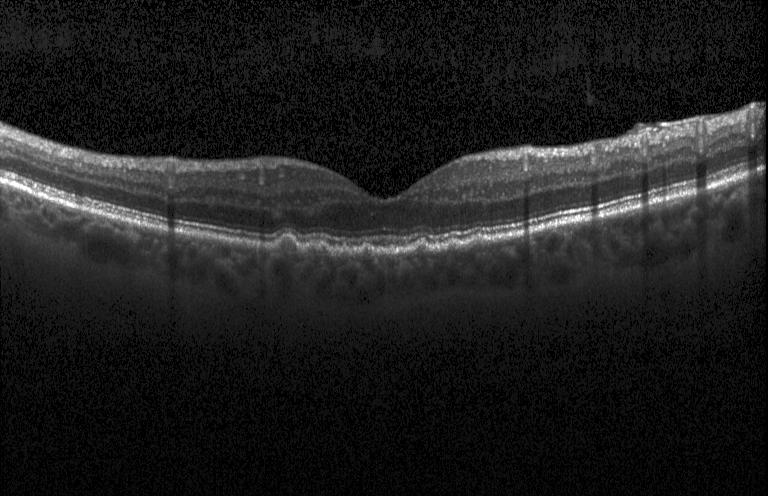

Optical coherence tomography scan; acquired on a Heidelberg Spectralis; spectral-domain optical coherence tomography — Impression: drusen.